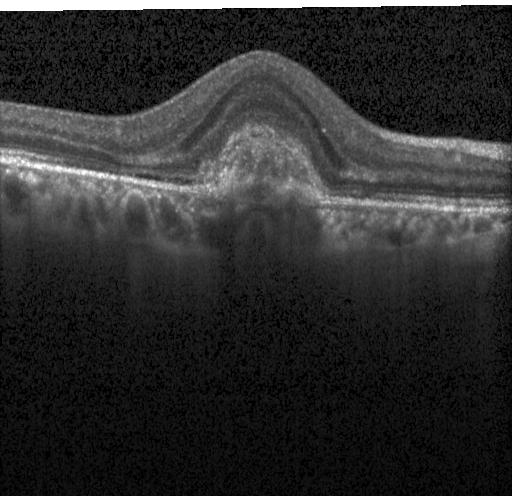
Heidelberg Spectralis OCT system, SD-OCT, OCT B-scan
Impression: CNV.